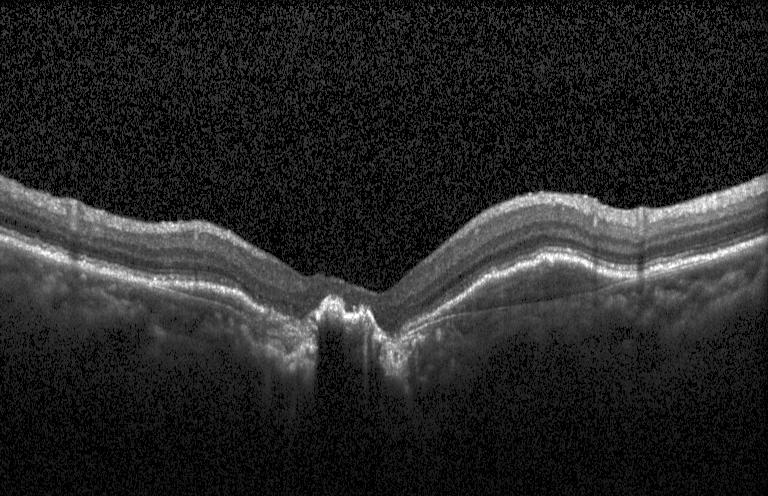

OCT B-scan — OCT finding: choroidal neovascularization (CNV).